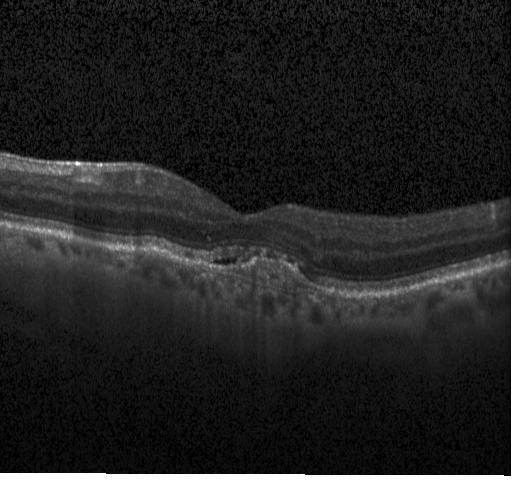 This B-scan demonstrates CNV.